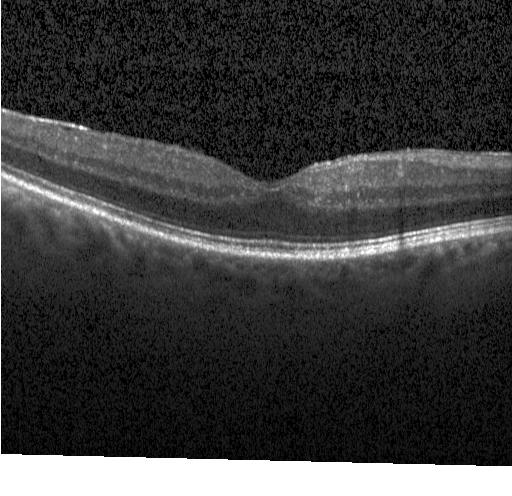
Retinal OCT cross-section showing no choroidal neovascularization, diabetic macular edema, or drusen.